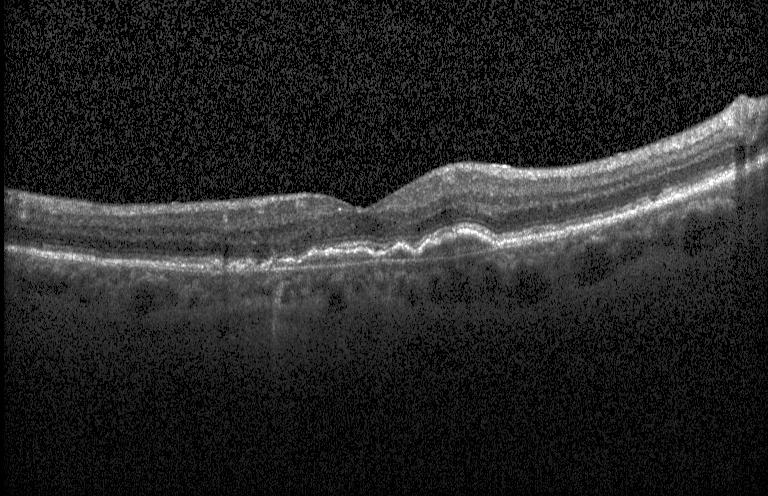
Optical coherence tomography B-scan. Assessment: a choroidal neovascular membrane.